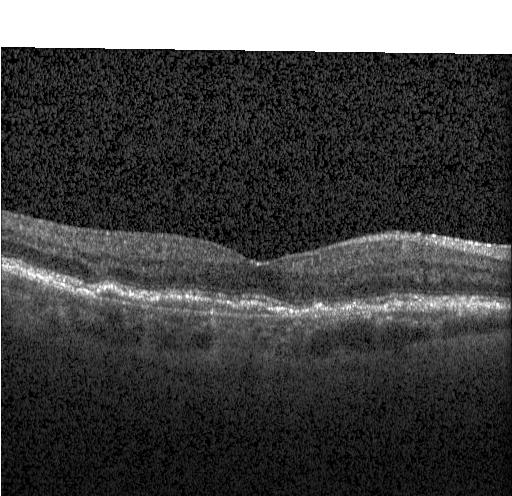
Retinal OCT B-scan. Dx: choroidal neovascularization (CNV).